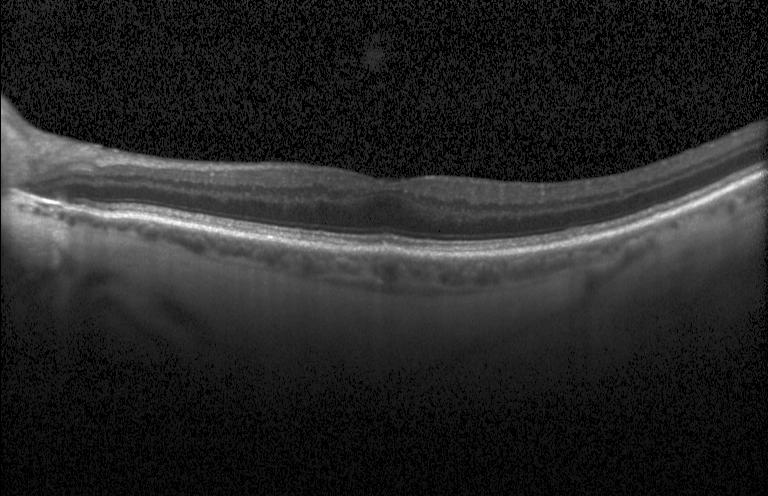 Assessment: no choroidal neovascularization, no diabetic macular edema, and no drusen.